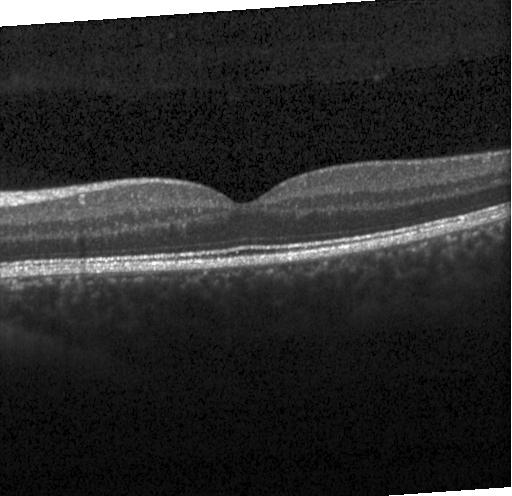 Finding: no choroidal neovascularization, diabetic macular edema, or drusen.